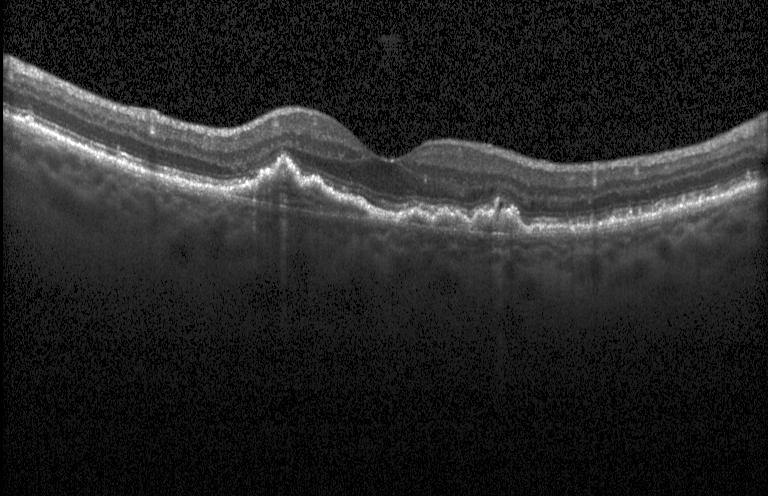

Diagnosis: choroidal neovascularization (CNV).